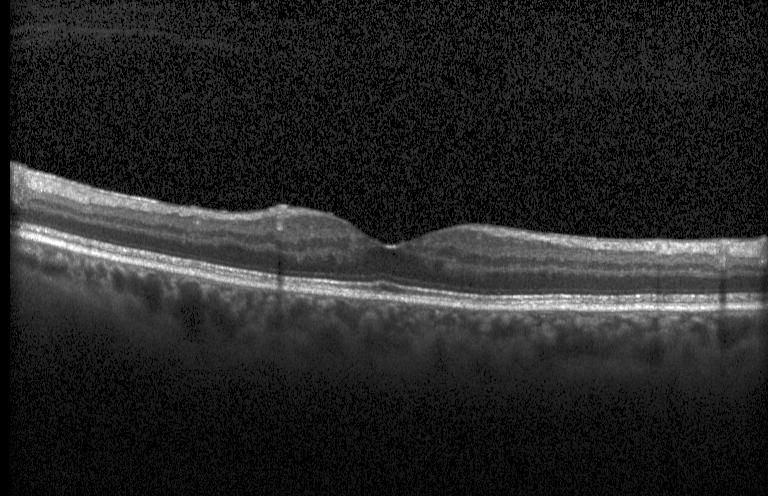

Optical coherence tomography scan; through the macula. Diagnosis: no evidence of choroidal neovascularization, diabetic macular edema, or drusen.